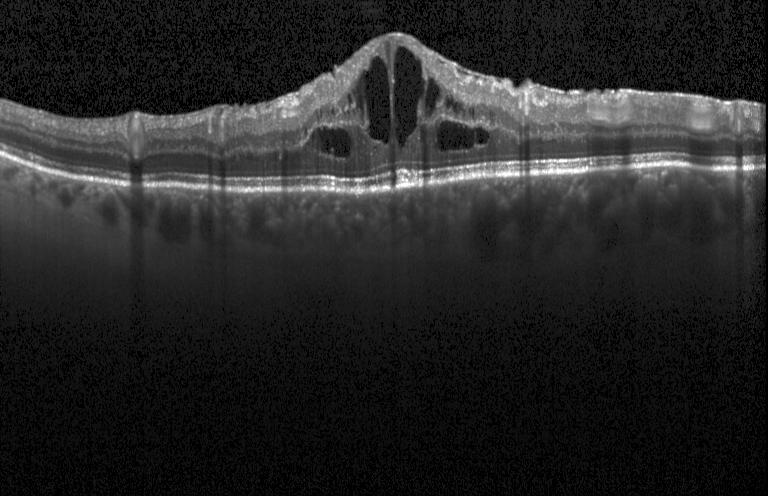
Optical coherence tomography scan. Heidelberg Spectralis. SD-OCT. Horizontal scan through the fovea. Macular OCT: DME.